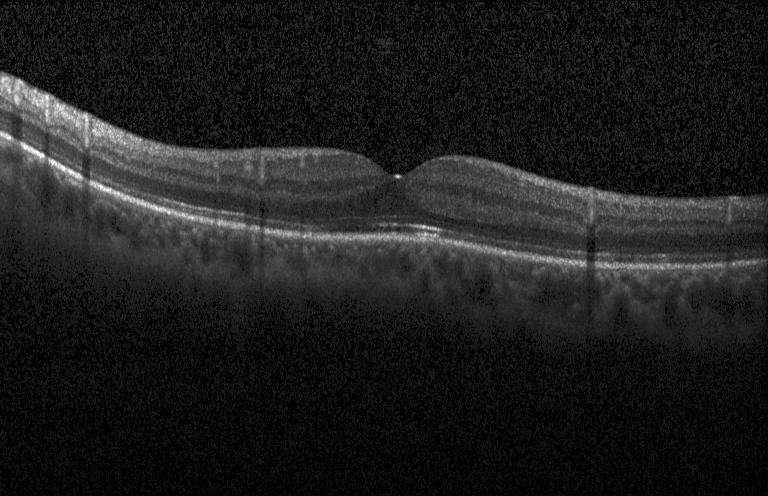 Assessment: neither choroidal neovascularization, diabetic macular edema, nor drusen.